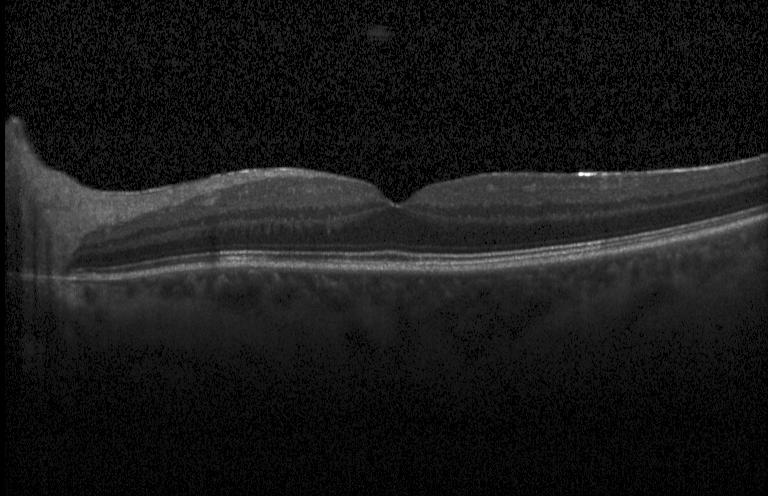
Heidelberg Spectralis. Spectral-domain optical coherence tomography. OCT line scan. Macular OCT: no choroidal neovascularization, no diabetic macular edema, and no drusen.